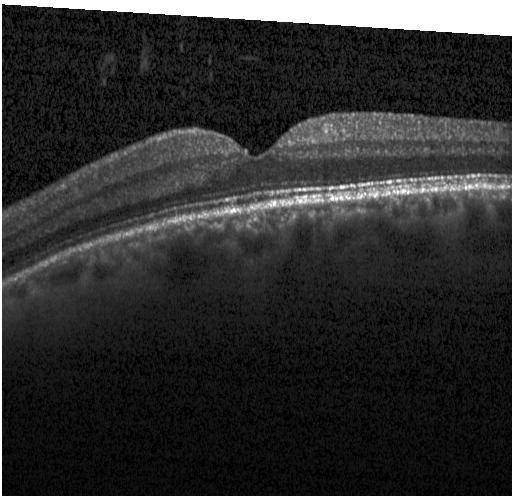

Spectral-domain optical coherence tomography; OCT B-scan — Impression: no CNV, DME, or drusen.